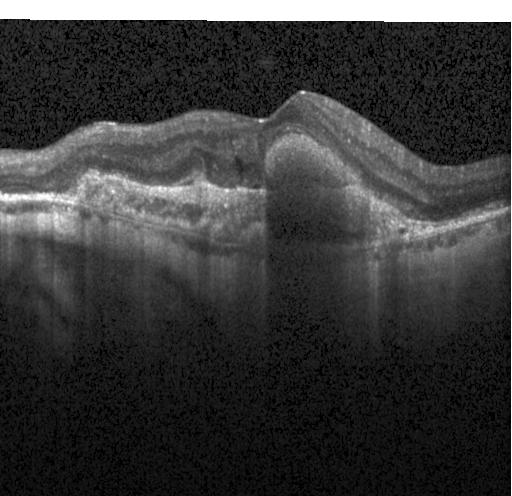
OCT B-scan, through the macula, spectral-domain OCT
Impression: a choroidal neovascular membrane.